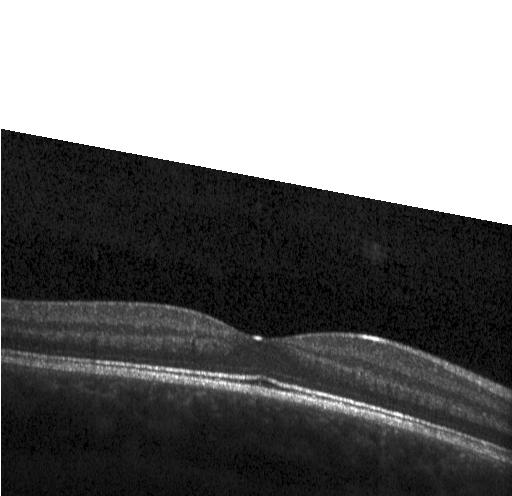

Impression: no CNV, no DME, and no drusen.